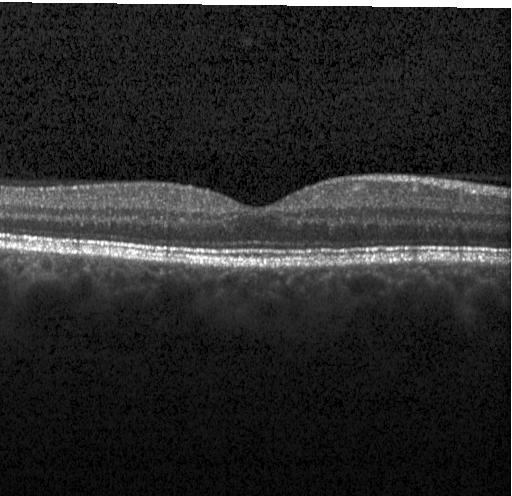
Acquired on a Heidelberg Spectralis, OCT line scan, spectral-domain optical coherence tomography
Impression: no choroidal neovascularization, diabetic macular edema, or drusen.